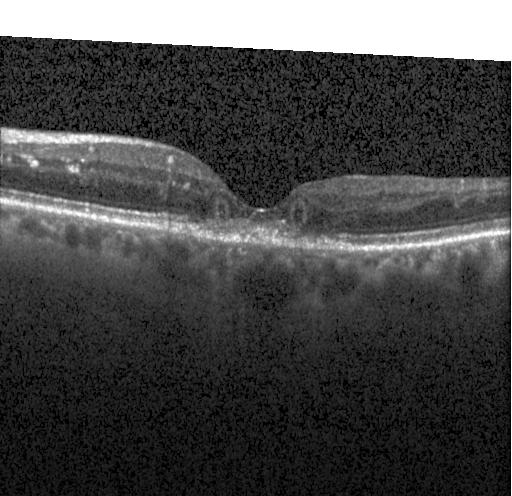

Retinal OCT cross-section, fovea-centered, acquired on a Heidelberg Spectralis, spectral-domain OCT.
This B-scan demonstrates choroidal neovascularization (CNV).